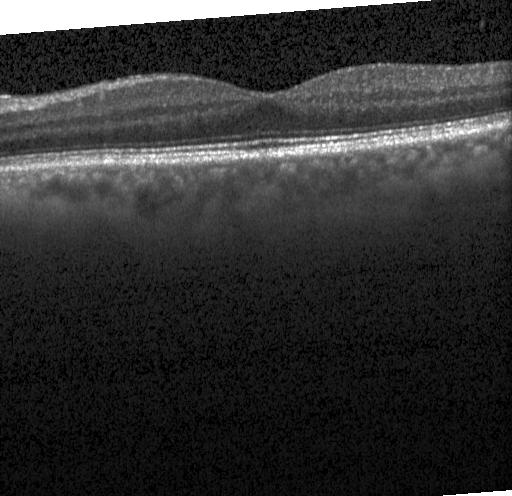

This B-scan demonstrates no CNV, DME, or drusen.